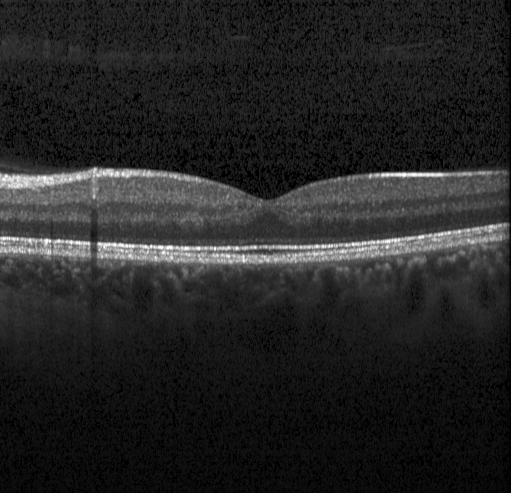
SD-OCT. Optical coherence tomography B-scan. Finding: neither CNV, DME, nor drusen.